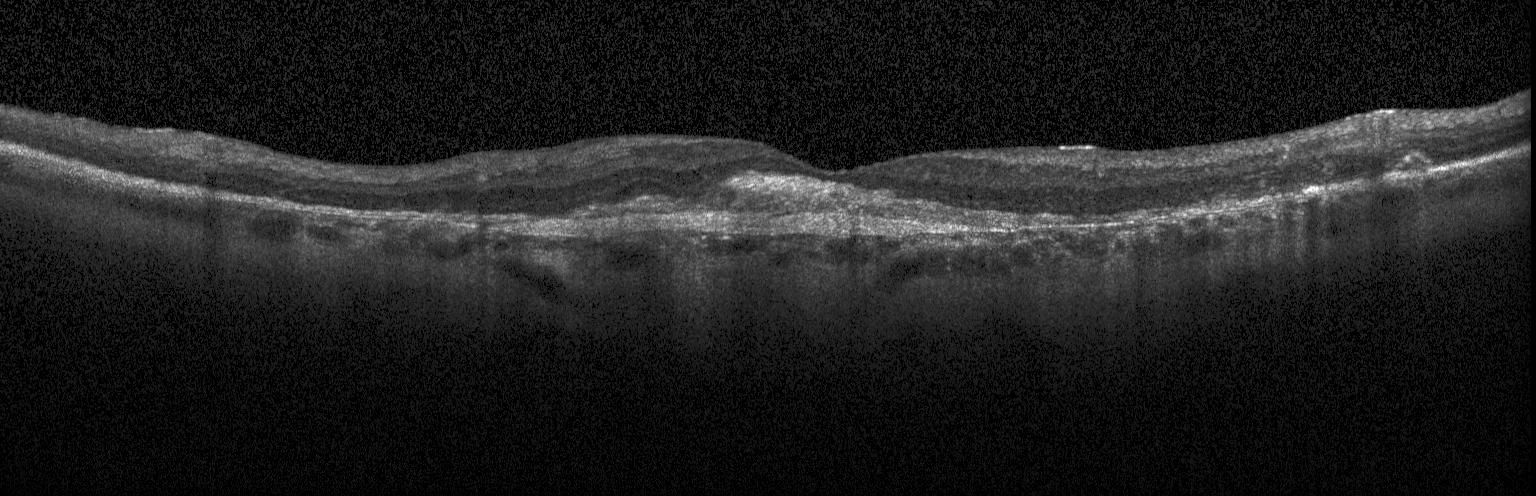
SD-OCT; instrument: Heidelberg Spectralis; retinal OCT B-scan; macular scan.
Impression: a choroidal neovascular membrane.